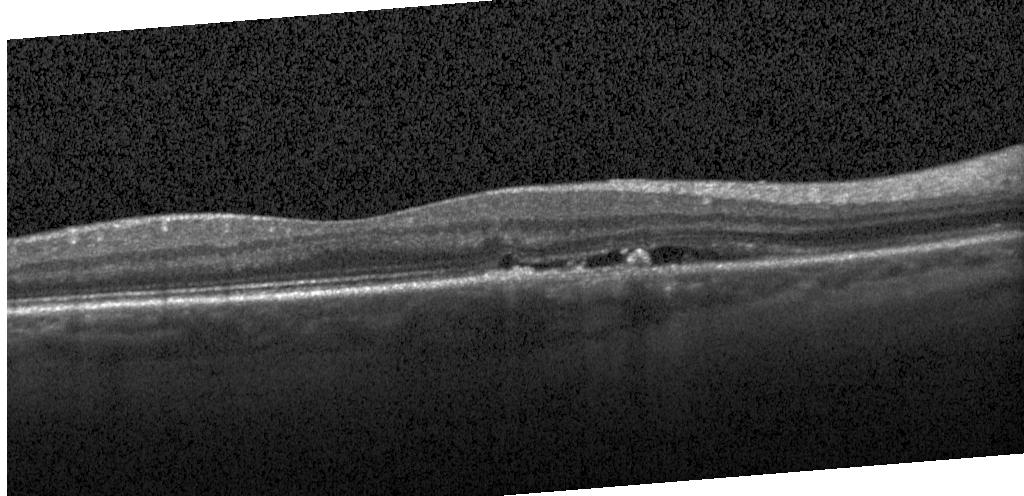 Heidelberg Spectralis OCT system, spectral-domain optical coherence tomography, optical coherence tomography B-scan.
A choroidal neovascular membrane.